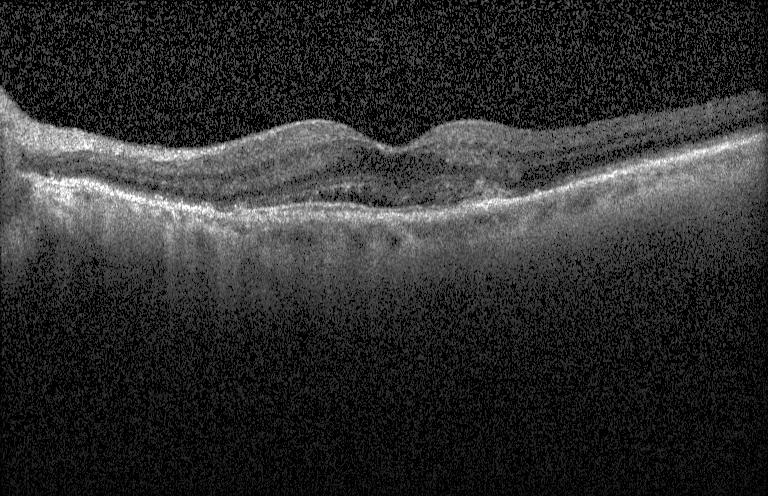
Optical coherence tomography scan. Impression: a choroidal neovascular membrane.